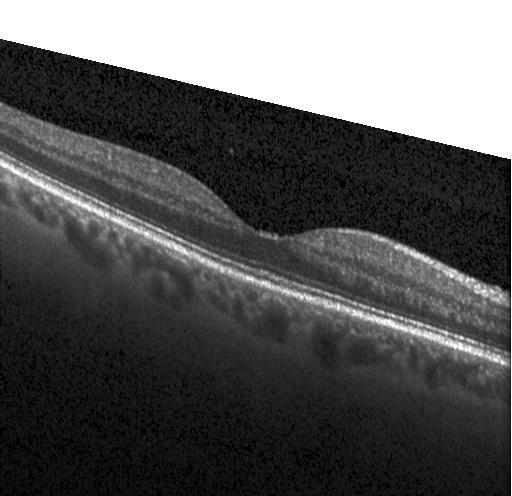
Macular scan · retinal OCT cross-section.
Macular OCT: neither choroidal neovascularization, diabetic macular edema, nor drusen.